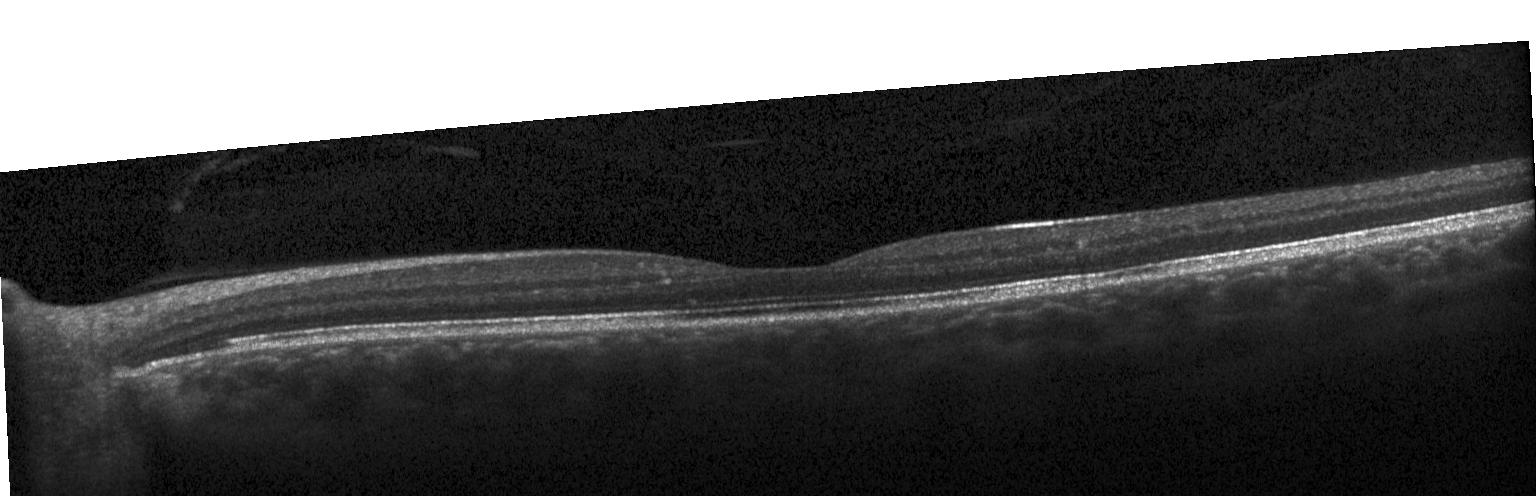 OCT scan showing neither CNV, DME, nor drusen.